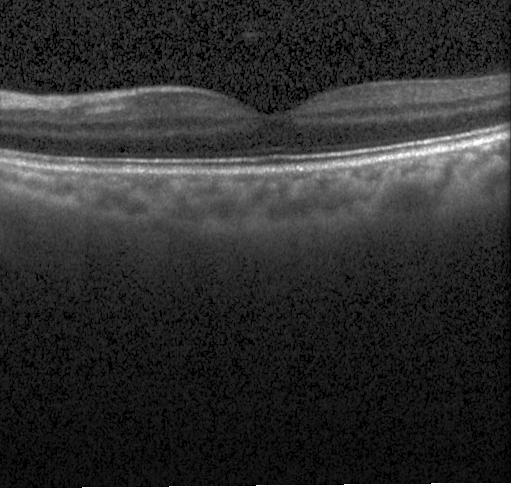
Heidelberg Spectralis OCT system; spectral-domain OCT; optical coherence tomography B-scan; macular scan. Impression: no CNV, DME, or drusen.